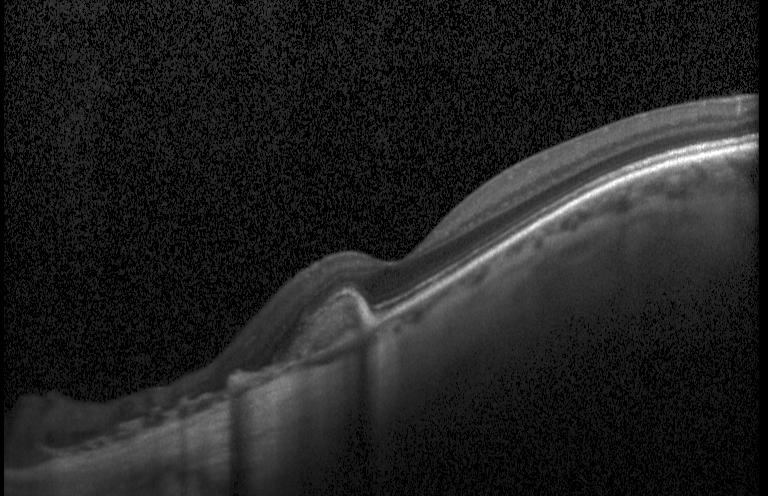
Heidelberg Spectralis, retinal OCT cross-section, horizontal scan through the fovea — Diagnosis: a choroidal neovascular membrane.